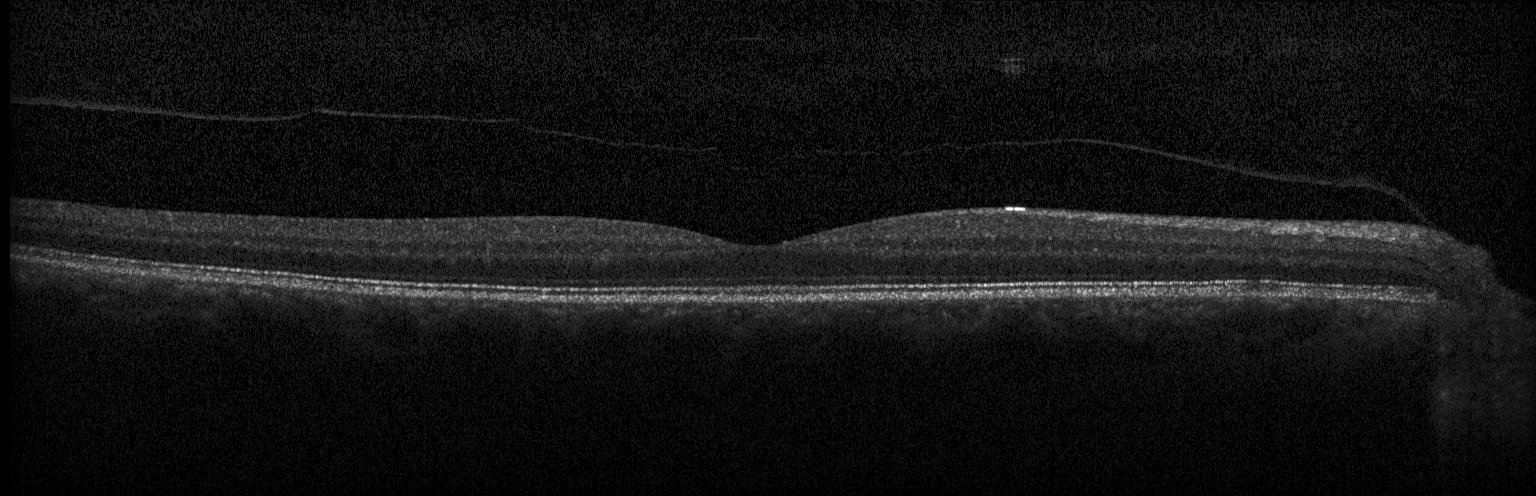
Heidelberg Spectralis OCT system · retinal OCT cross-section.
Dx: no evidence of choroidal neovascularization, diabetic macular edema, or drusen.